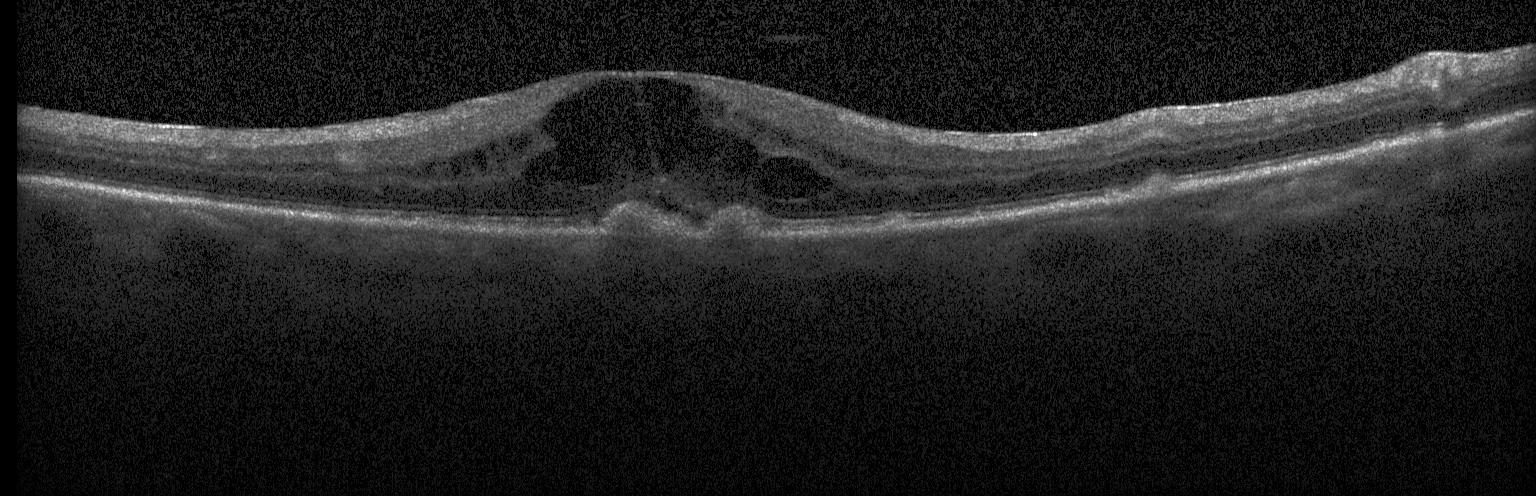 Heidelberg Spectralis OCT system; spectral-domain OCT; retinal OCT cross-section.
Impression: a choroidal neovascular membrane.